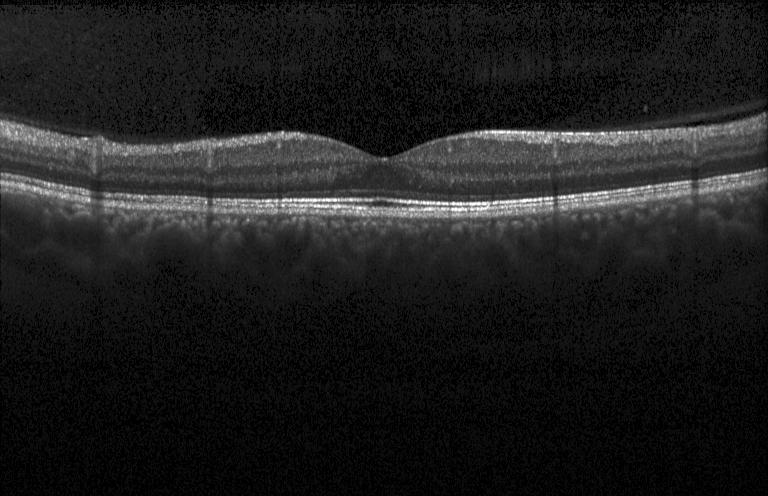 SD-OCT; optical coherence tomography scan; acquired on a Heidelberg Spectralis — Macular OCT: no choroidal neovascularization, no diabetic macular edema, and no drusen.